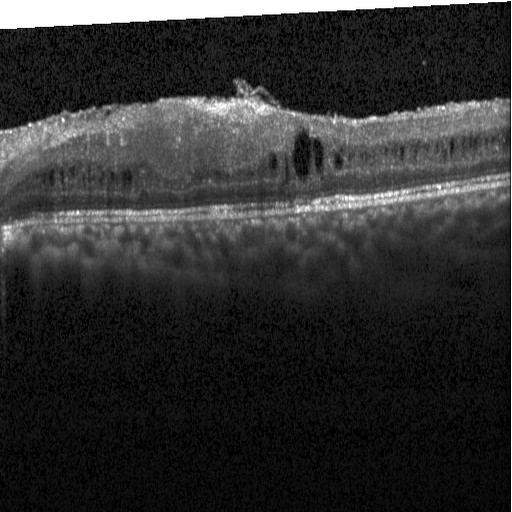

This B-scan demonstrates diabetic macular edema.